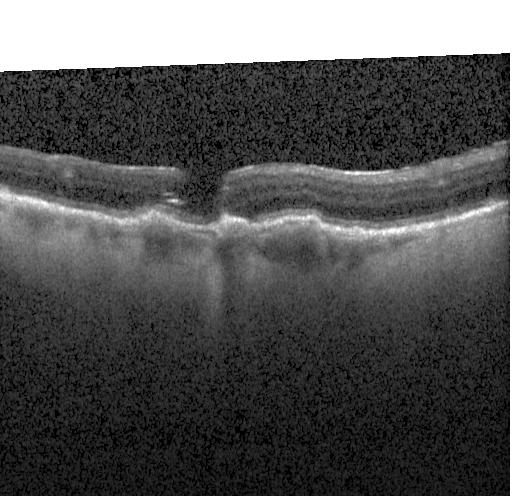 Dx: choroidal neovascularization (CNV).